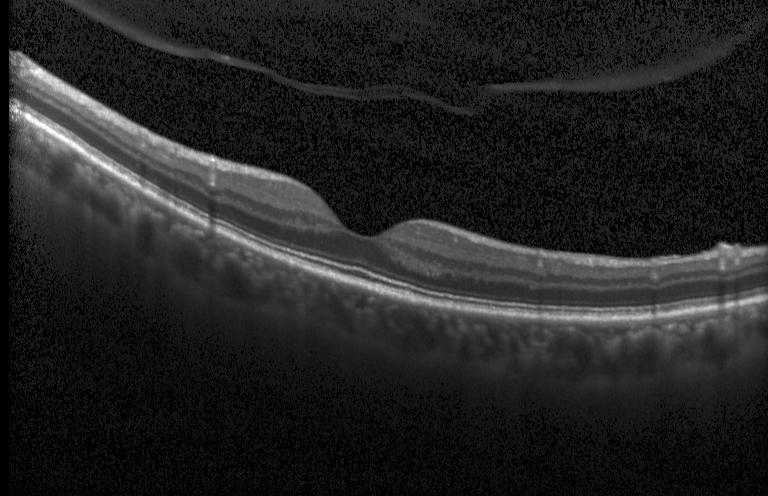

Diagnosis: no choroidal neovascularization, diabetic macular edema, or drusen.